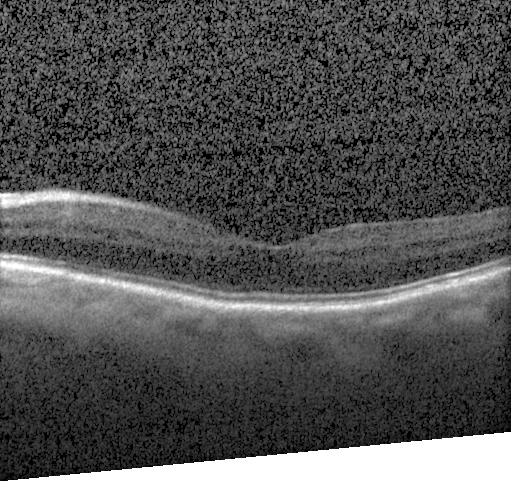 OCT line scan. Spectral-domain optical coherence tomography. Through the macula — This B-scan demonstrates no evidence of CNV, DME, or drusen.